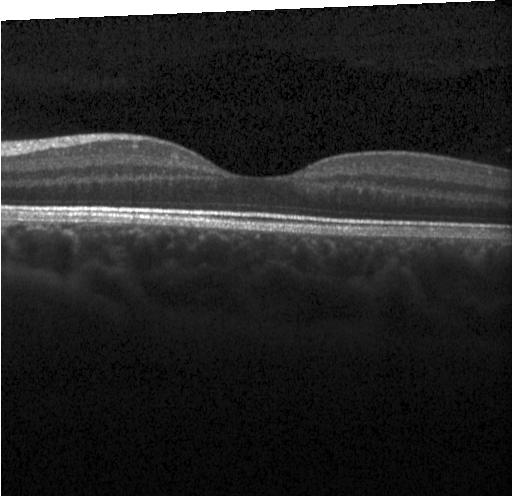 Dx: neither choroidal neovascularization, diabetic macular edema, nor drusen.